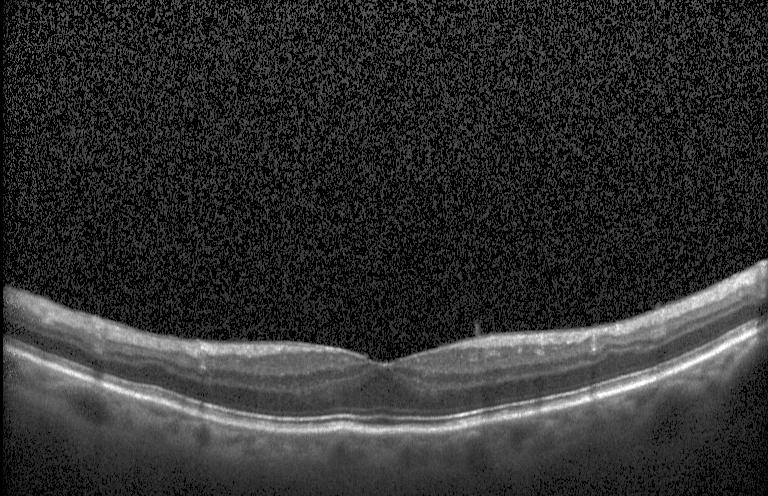
SD-OCT, OCT line scan
Assessment: no choroidal neovascularization, diabetic macular edema, or drusen.